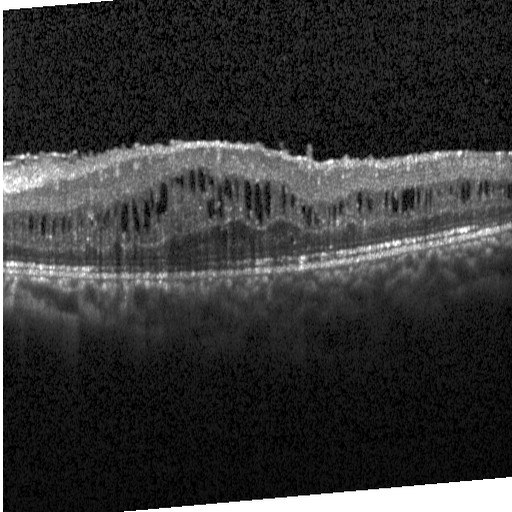

Optical coherence tomography B-scan. The scan shows diabetic macular edema.